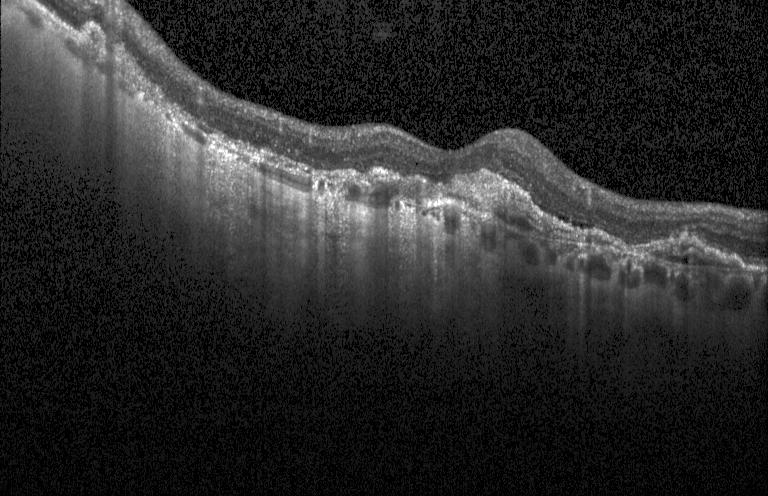 Optical coherence tomography scan; spectral-domain OCT.
Finding: choroidal neovascularization (CNV).